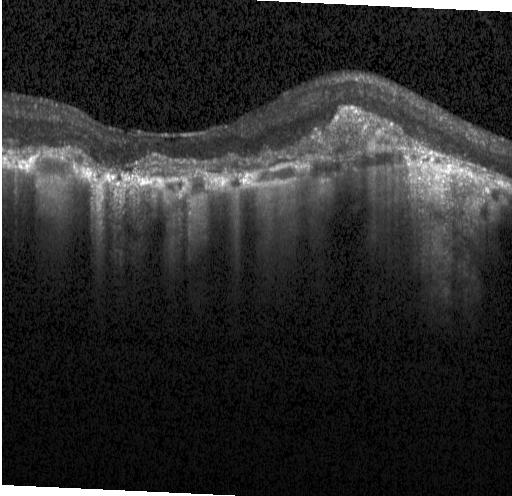

Optical coherence tomography B-scan. Macular scan. Heidelberg Spectralis. Spectral-domain optical coherence tomography.
Impression: a choroidal neovascular membrane.